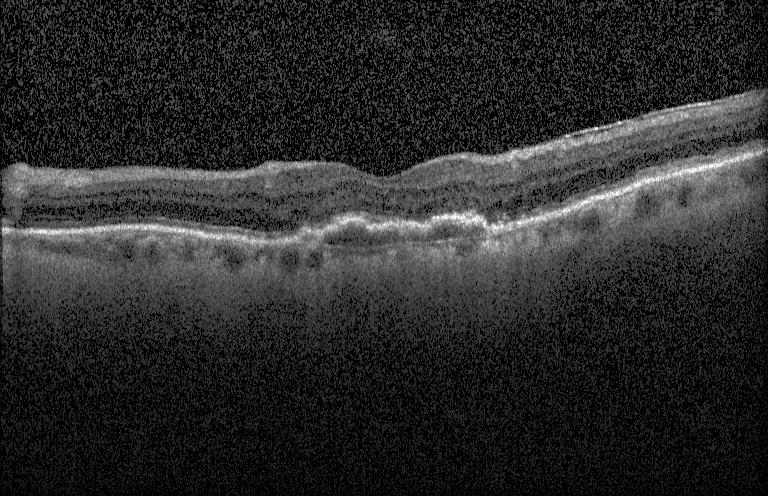 Retinal OCT B-scan
Diagnosis: a choroidal neovascular membrane.